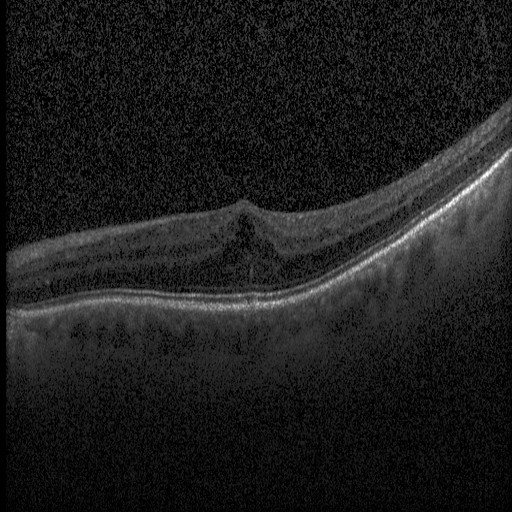
SD-OCT · retinal OCT B-scan — Macular OCT: diabetic macular edema.